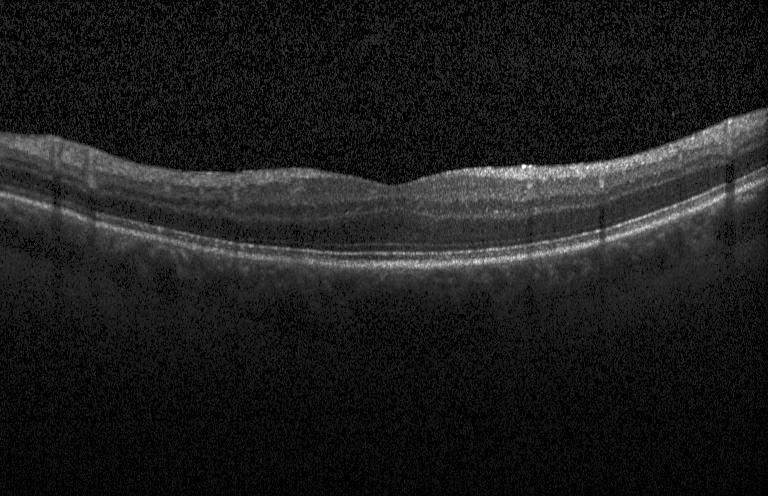
Macular OCT demonstrating no CNV, no DME, and no drusen.